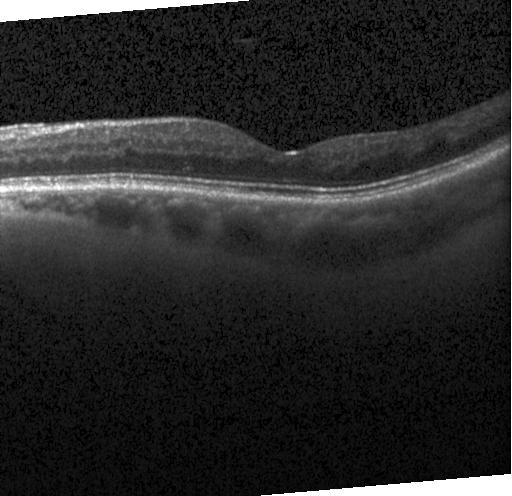

Retinal OCT B-scan, spectral-domain OCT, instrument: Heidelberg Spectralis. Assessment: no evidence of CNV, DME, or drusen.